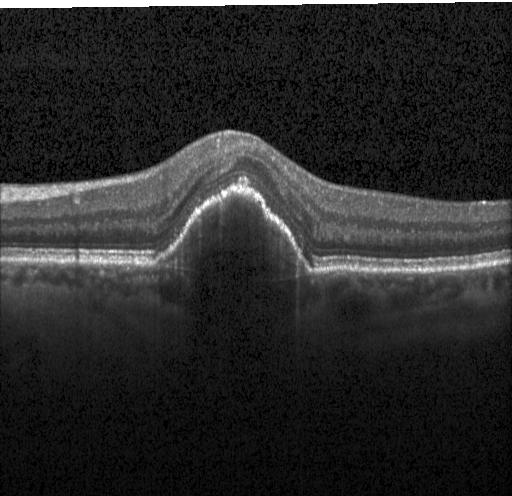
The scan shows choroidal neovascularization (CNV).